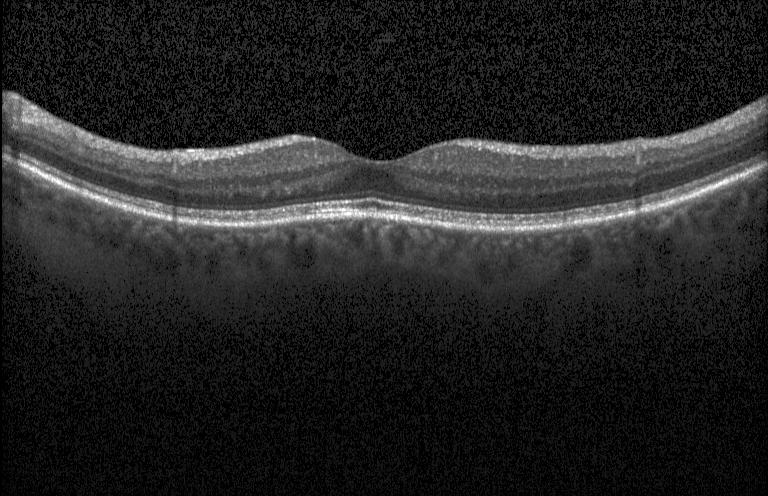
Optical coherence tomography B-scan; SD-OCT — The scan shows no choroidal neovascularization, diabetic macular edema, or drusen.